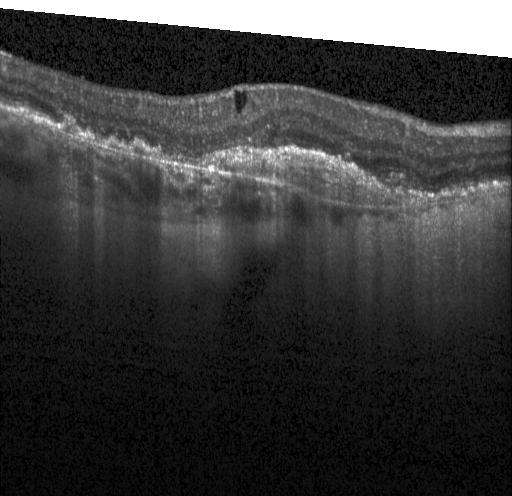
Optical coherence tomography B-scan, acquired on a Heidelberg Spectralis
Diagnosis: a choroidal neovascular membrane.